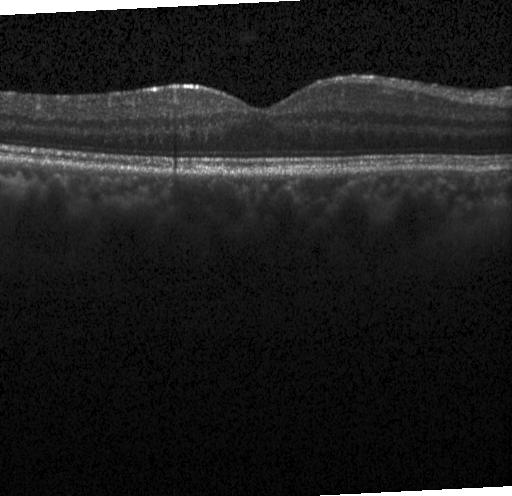
Retinal OCT B-scan · spectral-domain OCT — No evidence of CNV, DME, or drusen.